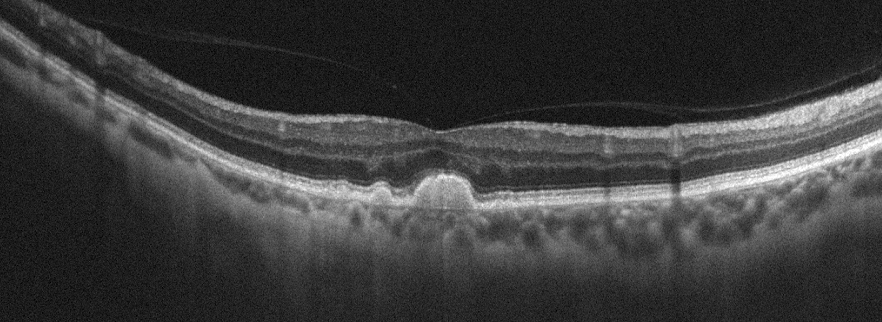
Retinal OCT cross-section. Right eye
The scan shows age-related macular degeneration.